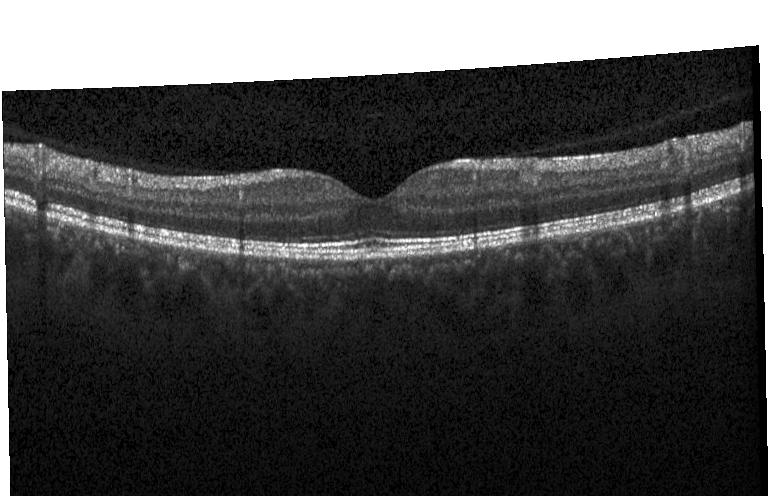

OCT line scan
No evidence of CNV, DME, or drusen.